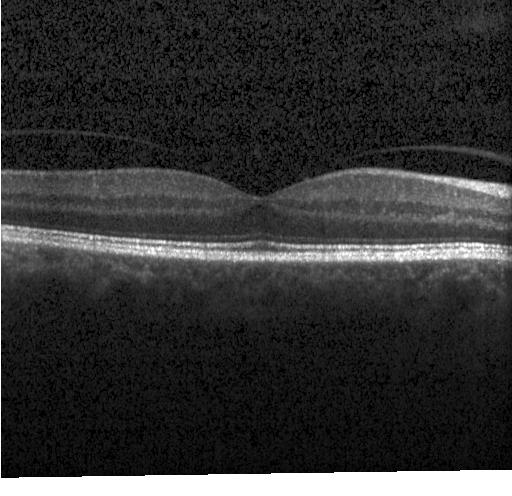

Instrument: Heidelberg Spectralis · optical coherence tomography B-scan. Impression: no choroidal neovascularization, no diabetic macular edema, and no drusen.